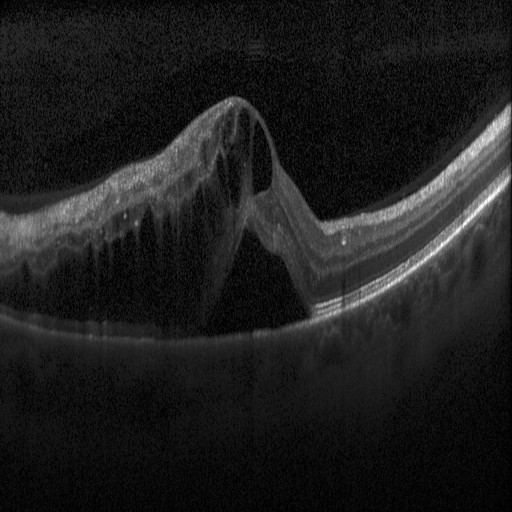
SD-OCT; instrument: Heidelberg Spectralis; retinal OCT B-scan; fovea-centered.
Diagnosis: DME.